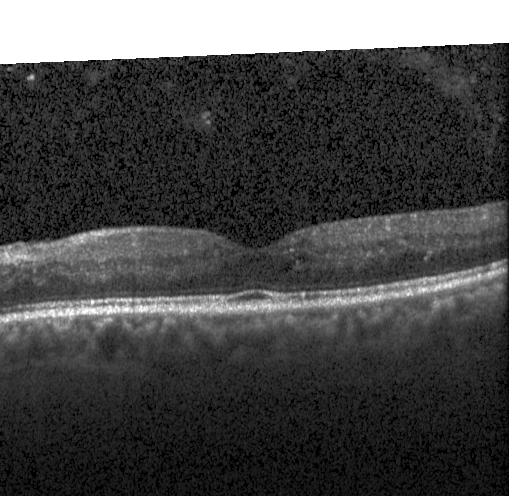

OCT finding: diabetic macular edema (DME).